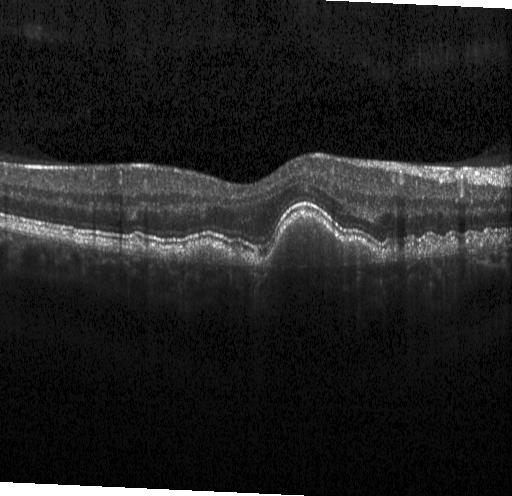 Spectral-domain optical coherence tomography · centered on the fovea · optical coherence tomography B-scan · Heidelberg Spectralis OCT system.
The scan shows drusen.